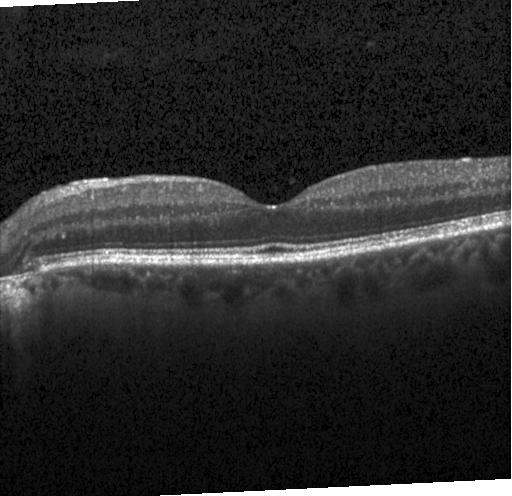

Impression: no evidence of choroidal neovascularization, diabetic macular edema, or drusen.